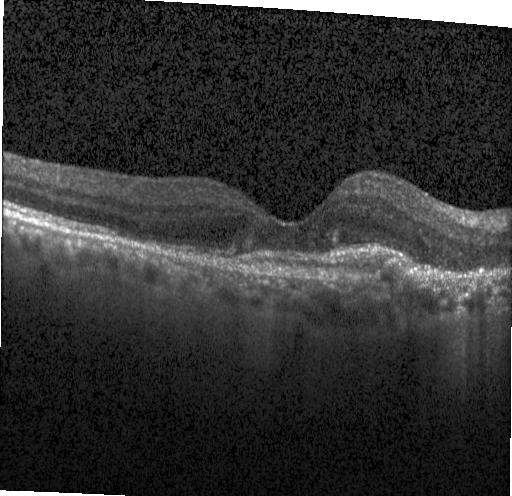
Optical coherence tomography scan.
Finding: choroidal neovascularization.